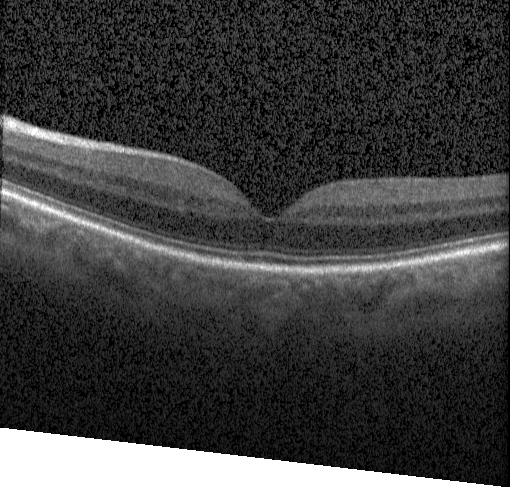

Spectral-domain optical coherence tomography, optical coherence tomography B-scan — The scan shows neither choroidal neovascularization, diabetic macular edema, nor drusen.